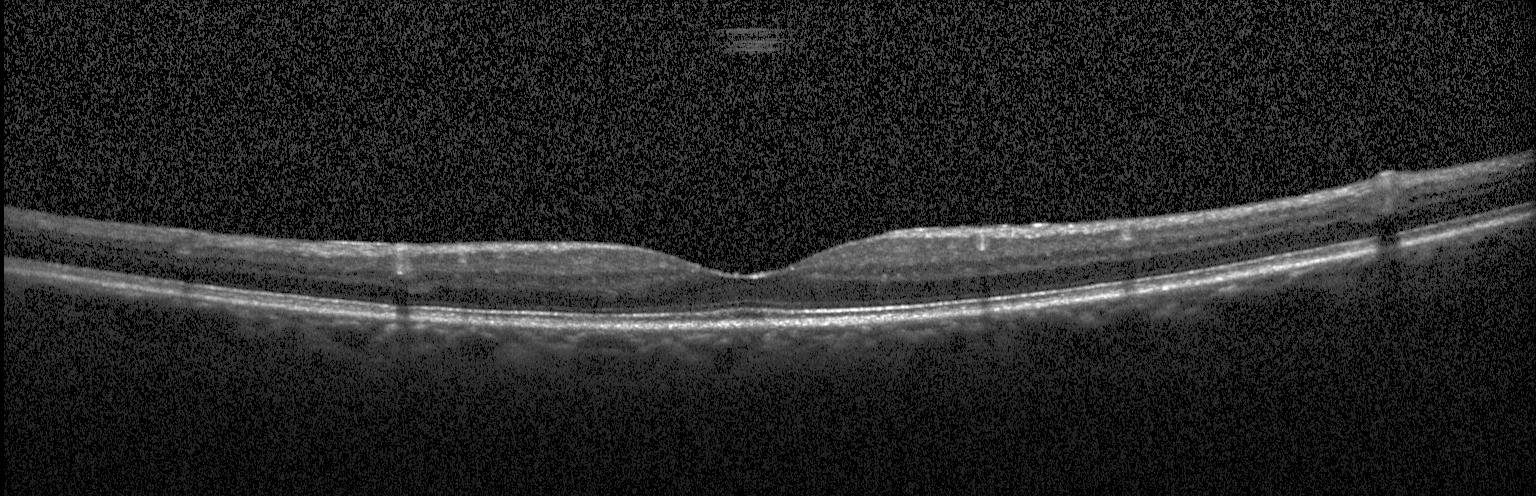

Spectral-domain OCT B-scan: no choroidal neovascularization, diabetic macular edema, or drusen.